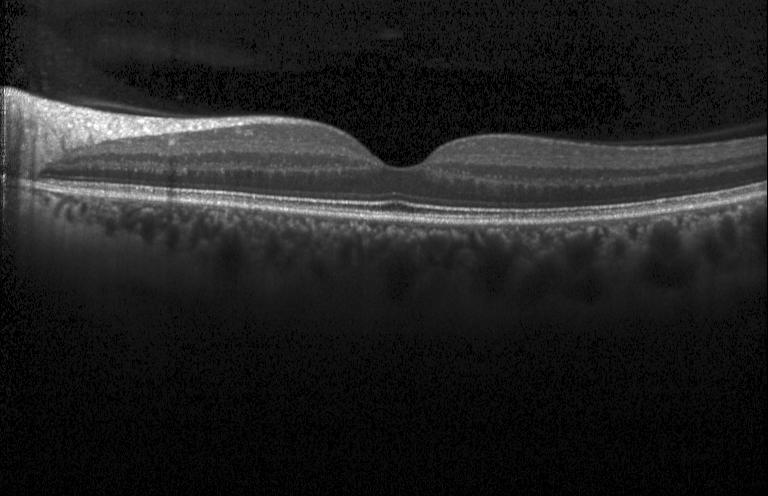
Heidelberg Spectralis; SD-OCT; optical coherence tomography B-scan; through the macula.
Impression: neither choroidal neovascularization, diabetic macular edema, nor drusen.